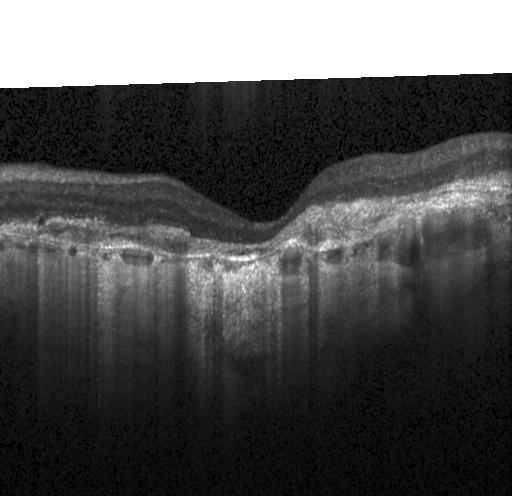

Spectral-domain OCT. OCT B-scan — Macular OCT: choroidal neovascularization (CNV).